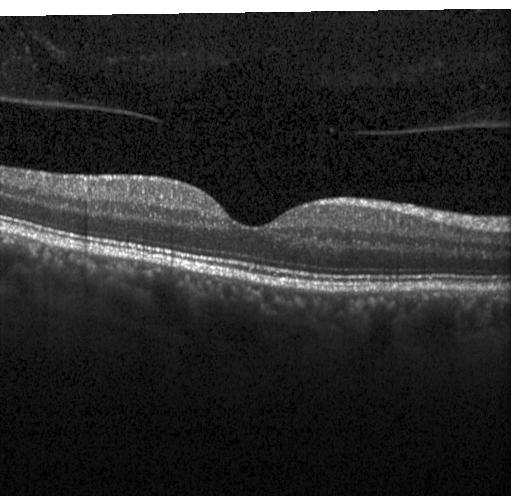

Spectral-domain optical coherence tomography; OCT B-scan; centered on the fovea — No choroidal neovascularization, no diabetic macular edema, and no drusen.